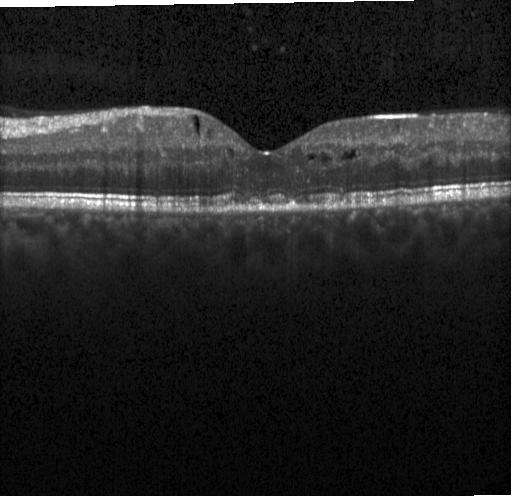
Diabetic macular edema.